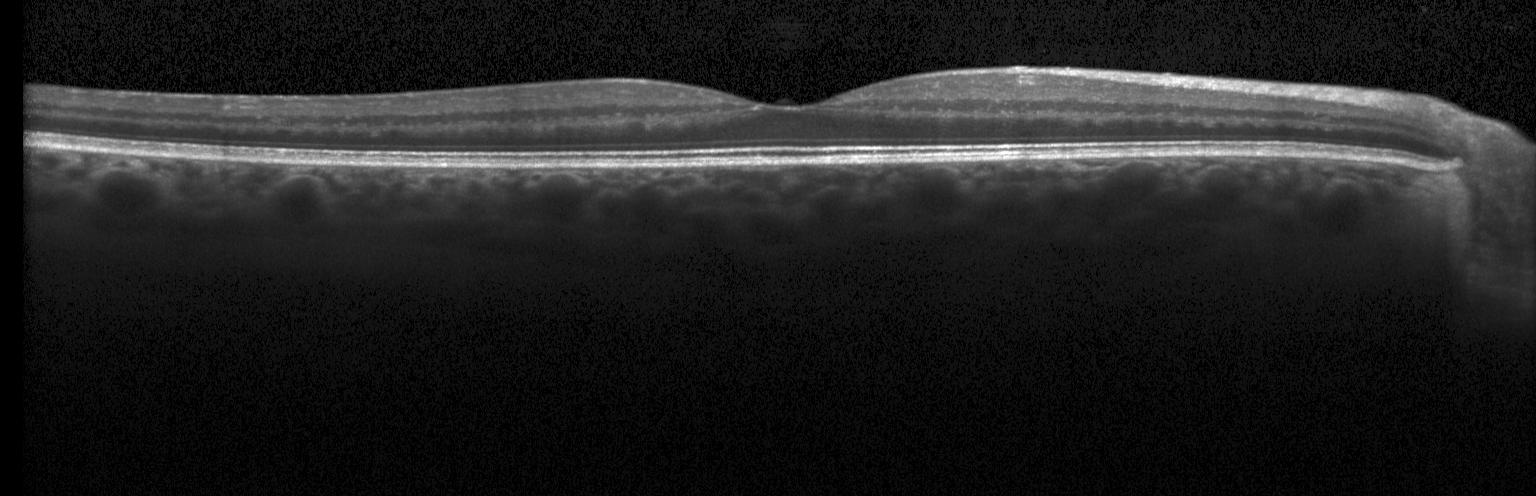
Horizontal scan through the fovea · OCT B-scan · Heidelberg Spectralis · SD-OCT
Diagnosis: neither CNV, DME, nor drusen.